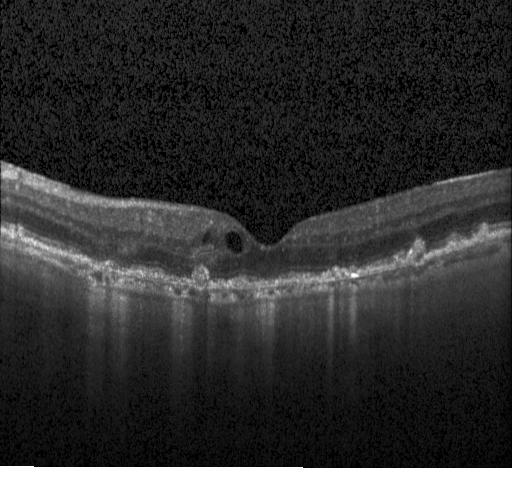

Diagnosis: a choroidal neovascular membrane.